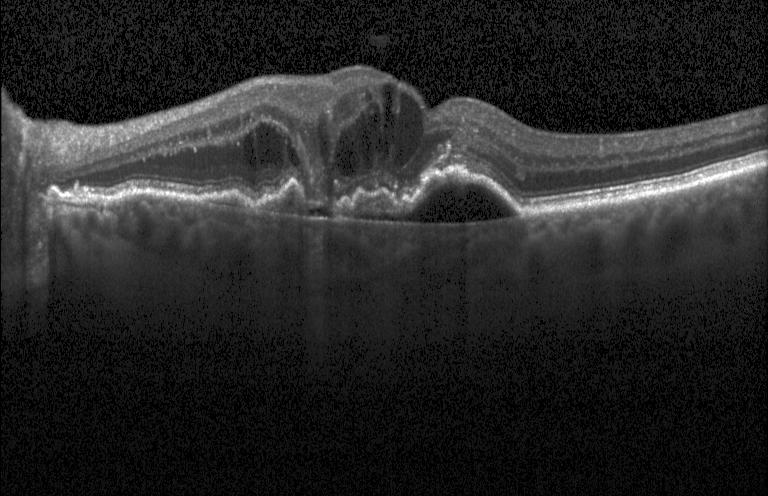
Assessment: choroidal neovascularization (CNV).